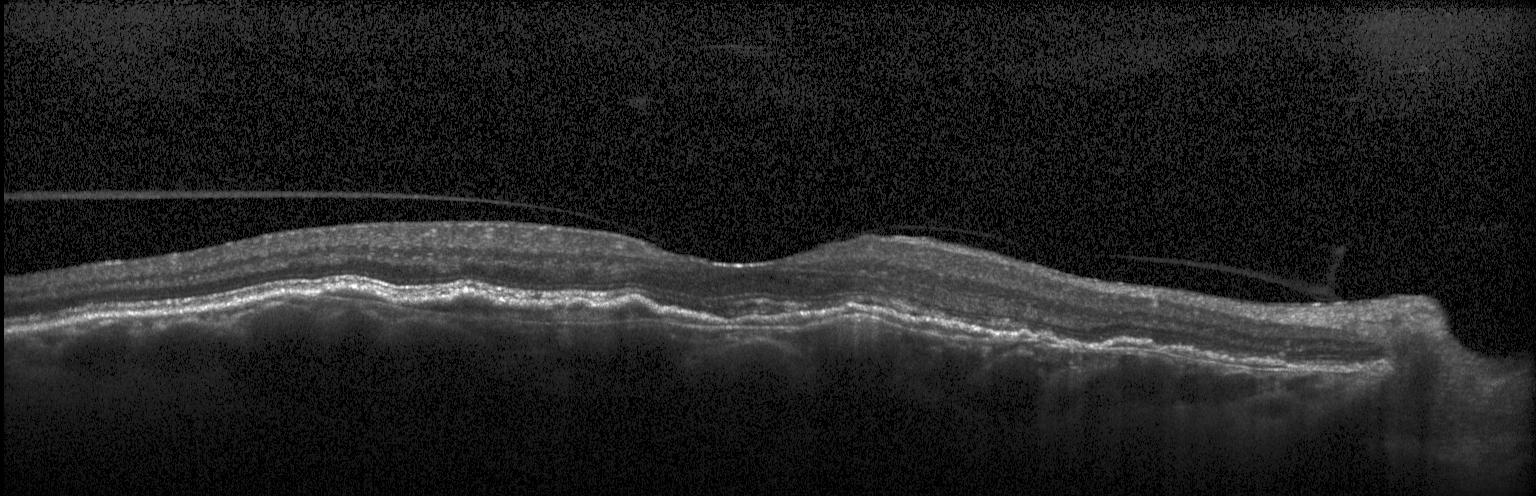

Optical coherence tomography B-scan. Impression: a choroidal neovascular membrane.